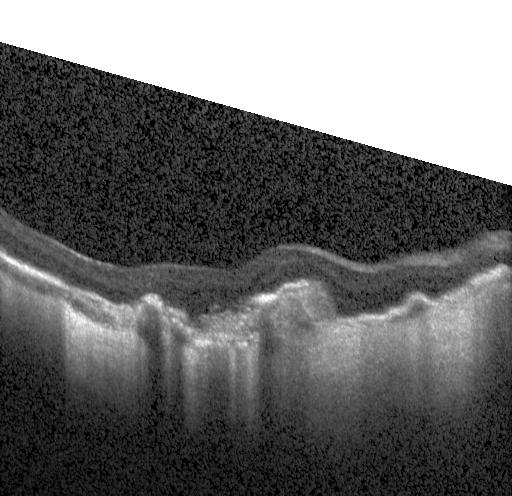
Diagnosis: CNV.